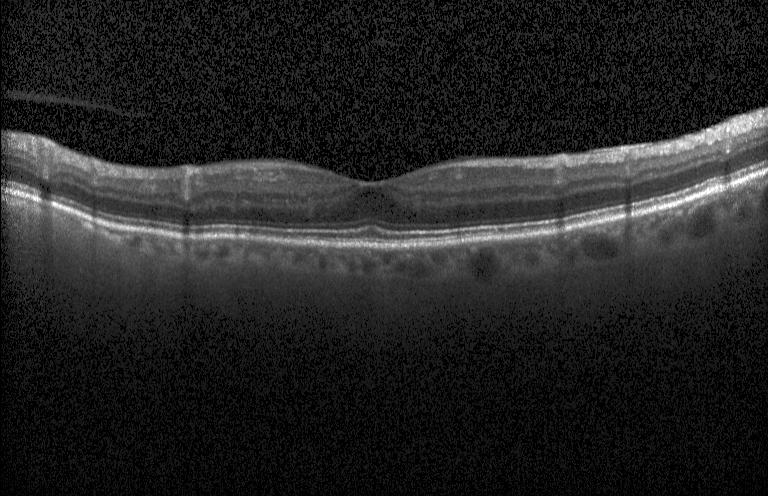 Spectral-domain optical coherence tomography; instrument: Heidelberg Spectralis; macular scan; retinal OCT cross-section
Macular OCT: no choroidal neovascularization, no diabetic macular edema, and no drusen.